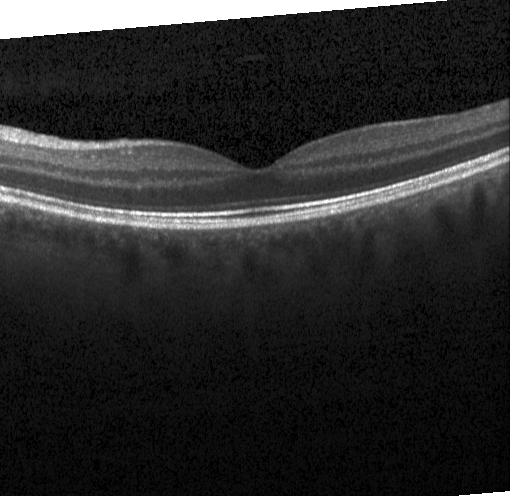
Retinal OCT cross-section · centered on the fovea · SD-OCT · acquired on a Heidelberg Spectralis
Diagnosis: no choroidal neovascularization, diabetic macular edema, or drusen.